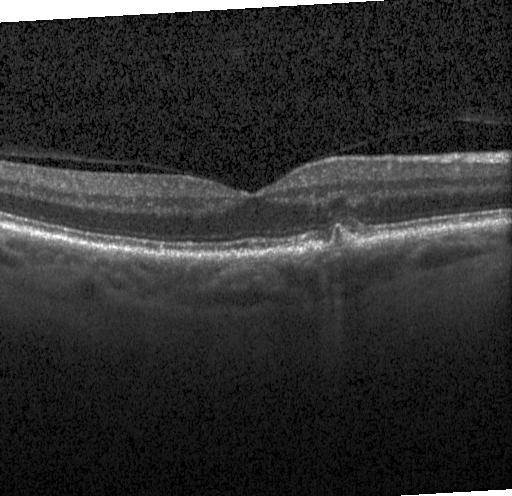

Macular OCT demonstrating multiple drusen.